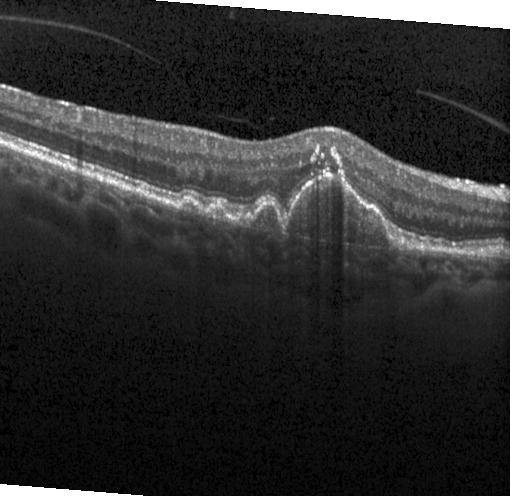
Retinal OCT cross-section, spectral-domain OCT — Dx: a choroidal neovascular membrane.